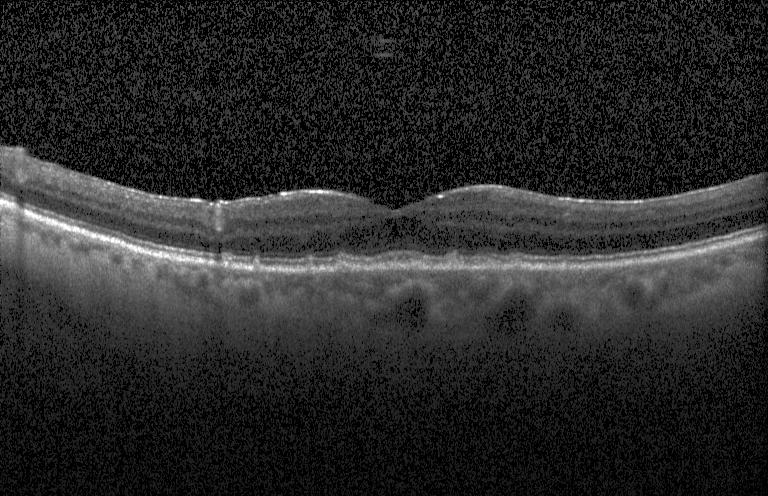

OCT line scan. Finding: multiple drusen.